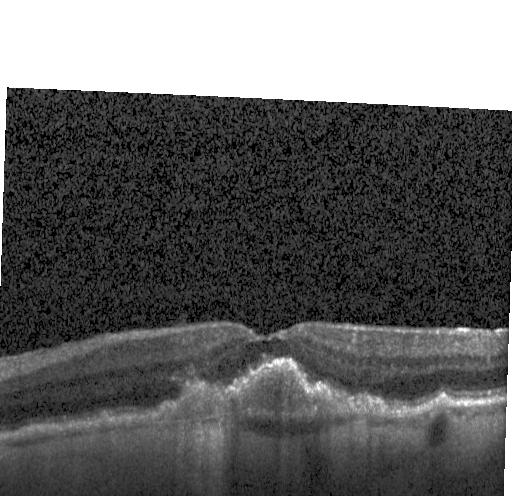

Fovea-centered. OCT B-scan. Impression: a choroidal neovascular membrane.